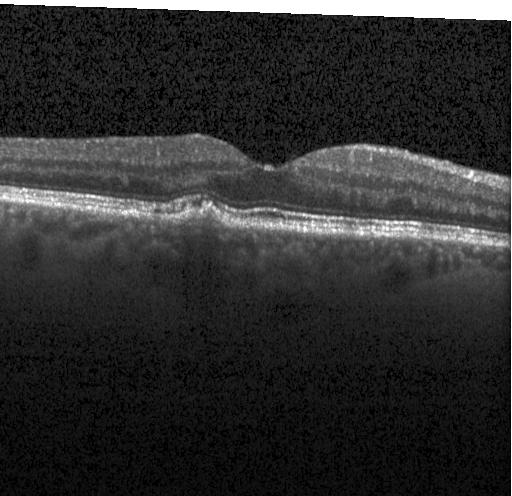
Diagnosis: multiple drusen.